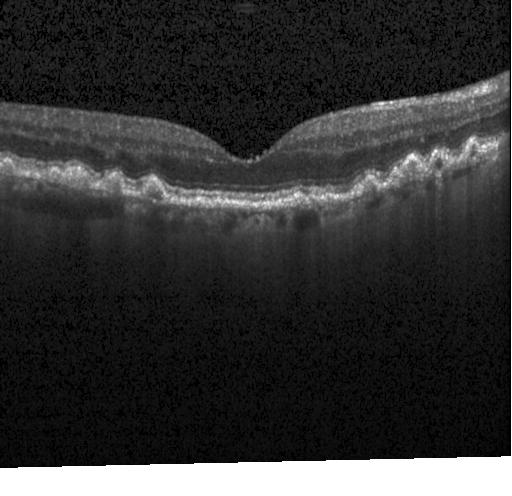 Heidelberg Spectralis; optical coherence tomography scan. Assessment: multiple drusen.